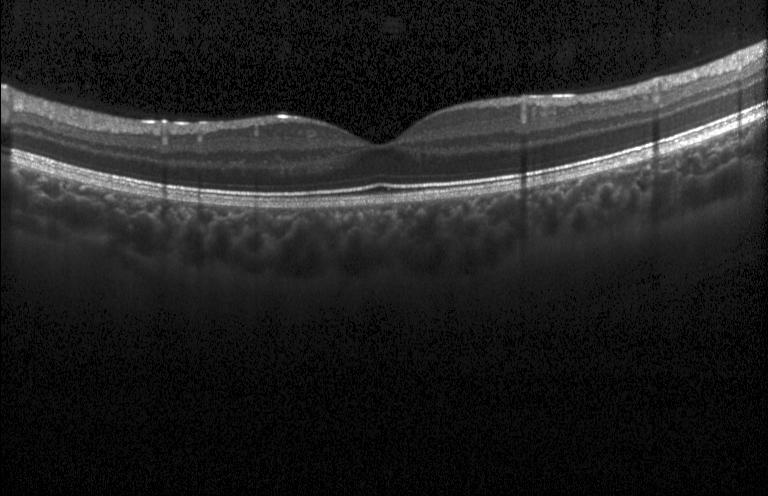

Assessment: neither CNV, DME, nor drusen.